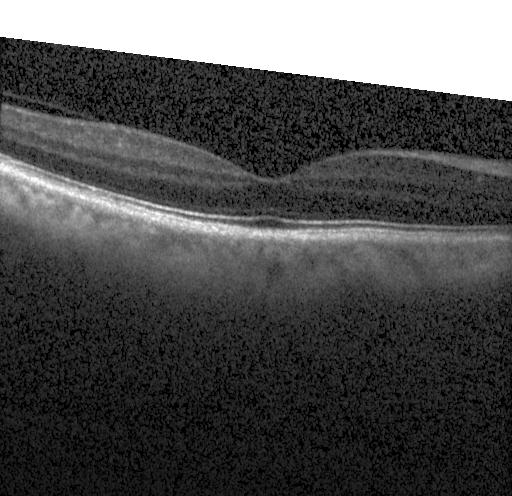
Instrument: Heidelberg Spectralis · OCT line scan — Impression: no CNV, DME, or drusen.